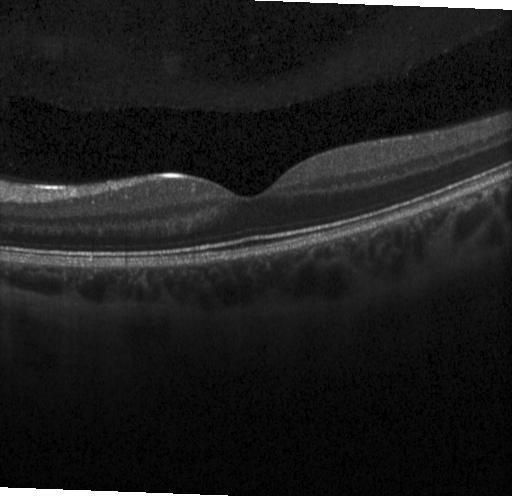 OCT finding: no choroidal neovascularization, no diabetic macular edema, and no drusen.